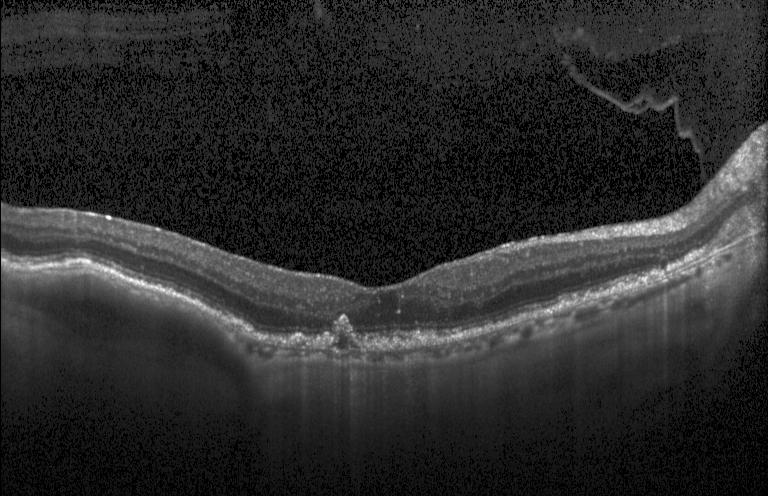 OCT scan showing a choroidal neovascular membrane.